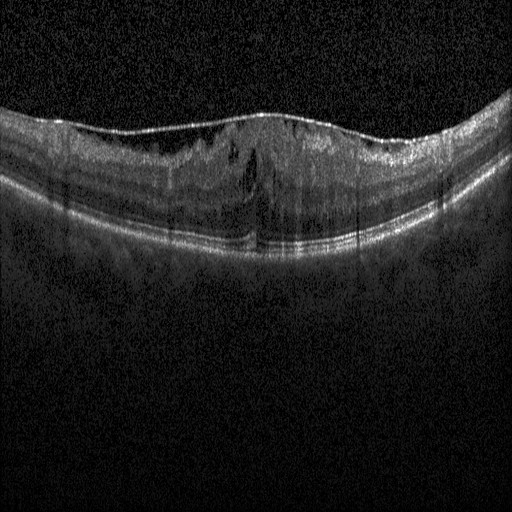

Centered on the fovea; OCT B-scan
Diagnosis: diabetic macular edema.